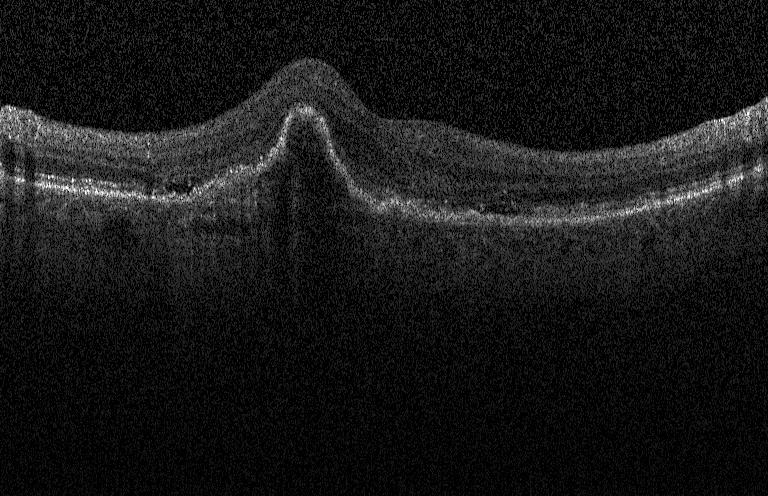
Centered on the fovea · OCT B-scan — Assessment: choroidal neovascularization.